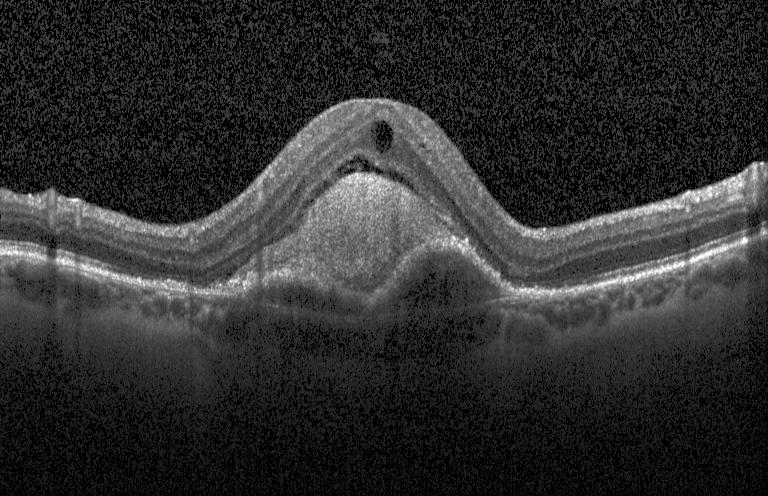

OCT B-scan — Dx: a choroidal neovascular membrane.